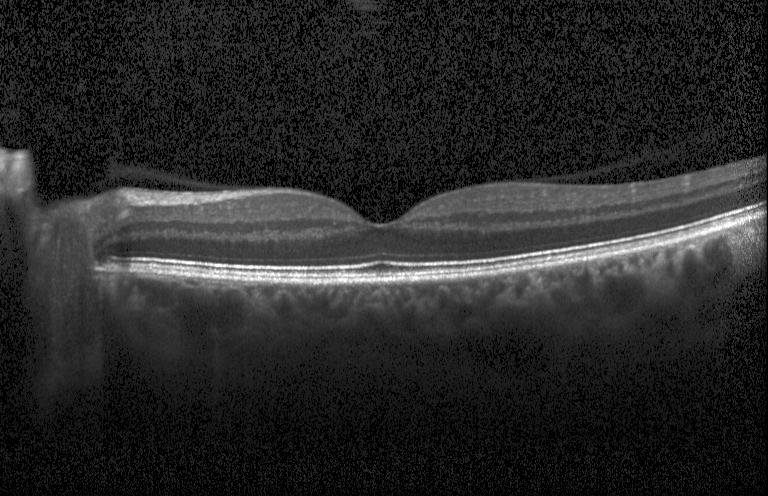 Macular OCT: no evidence of choroidal neovascularization, diabetic macular edema, or drusen.